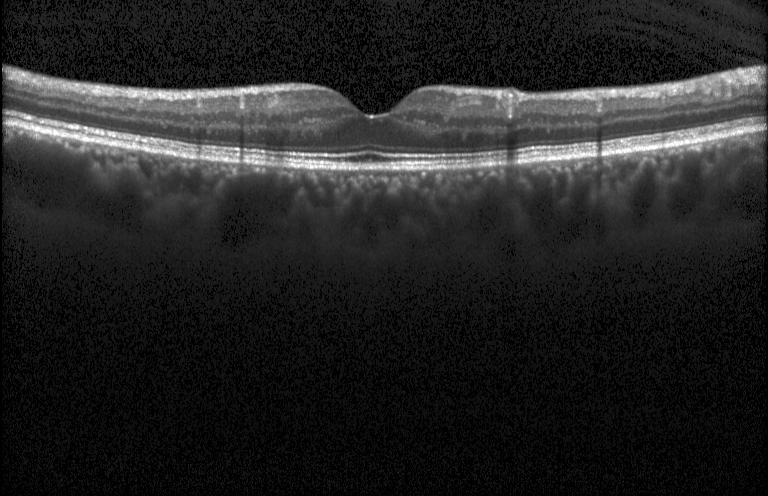

Impression: no choroidal neovascularization, diabetic macular edema, or drusen.